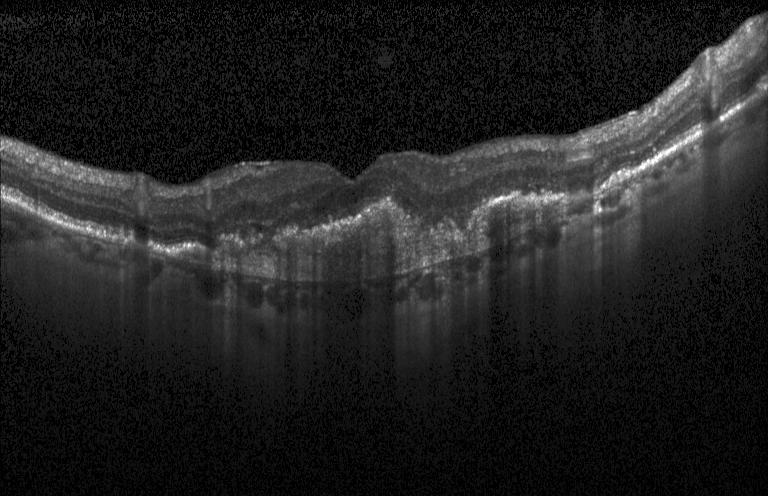

Optical coherence tomography B-scan. Heidelberg Spectralis. SD-OCT. Horizontal scan through the fovea
The scan shows a choroidal neovascular membrane.